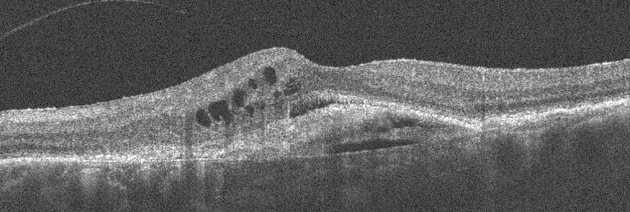
Retinal OCT B-scan · left eye
Age-related macular degeneration (AMD).